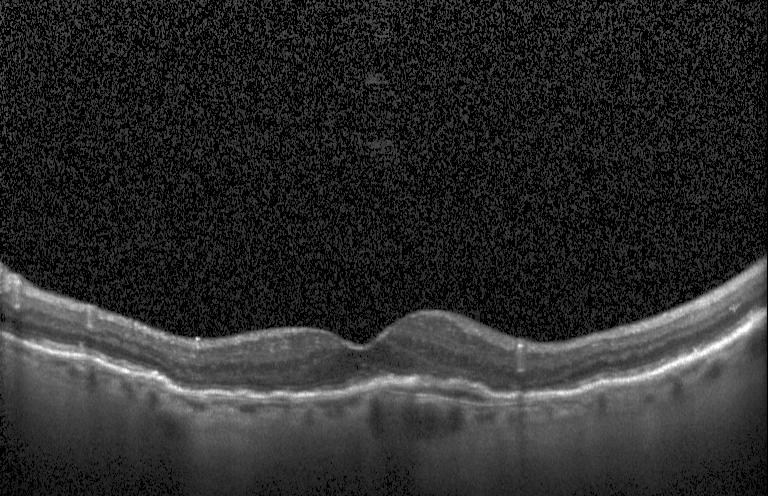 OCT line scan, through the macula. A choroidal neovascular membrane.